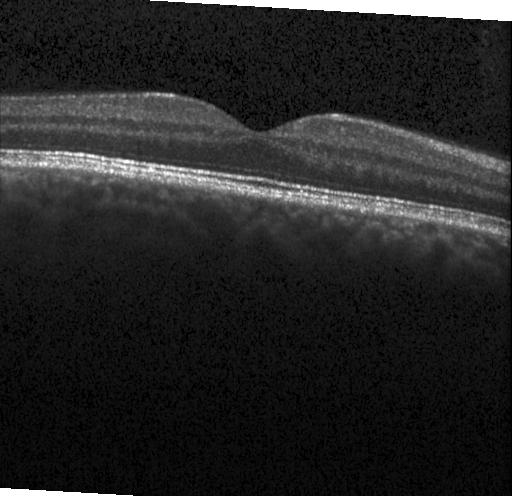
Optical coherence tomography B-scan — Finding: neither choroidal neovascularization, diabetic macular edema, nor drusen.